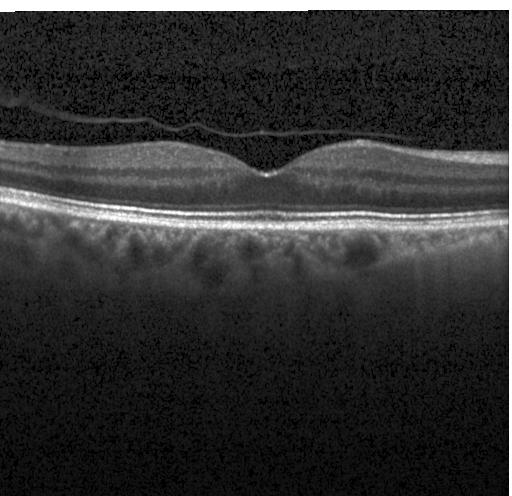
OCT B-scan.
Assessment: neither choroidal neovascularization, diabetic macular edema, nor drusen.